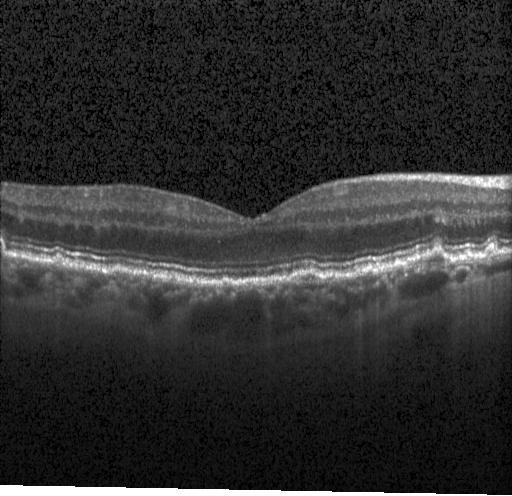 Optical coherence tomography B-scan
OCT finding: drusen.